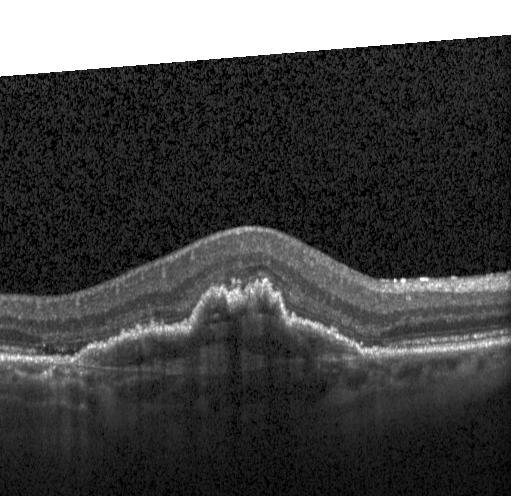 Finding: choroidal neovascularization (CNV).